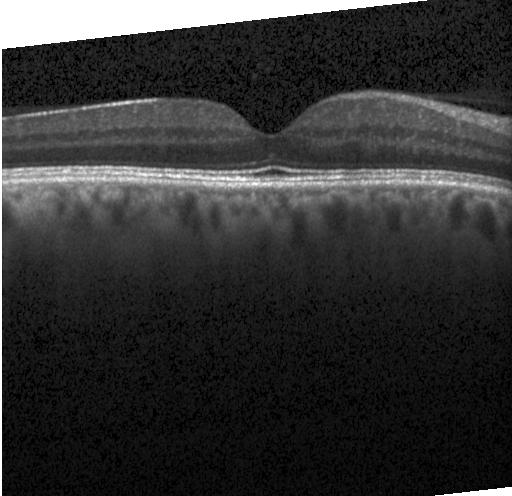 Macular OCT demonstrating no choroidal neovascularization, diabetic macular edema, or drusen.